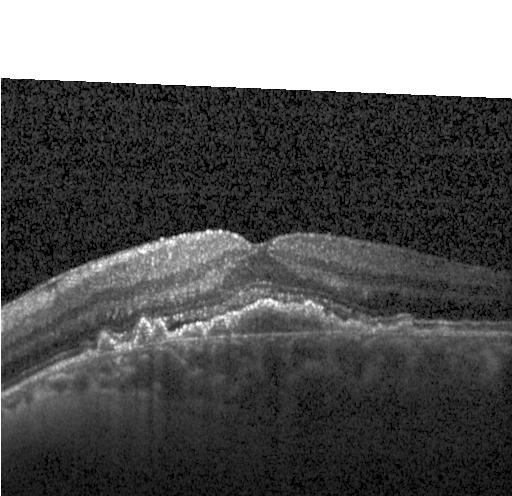
Impression: choroidal neovascularization.